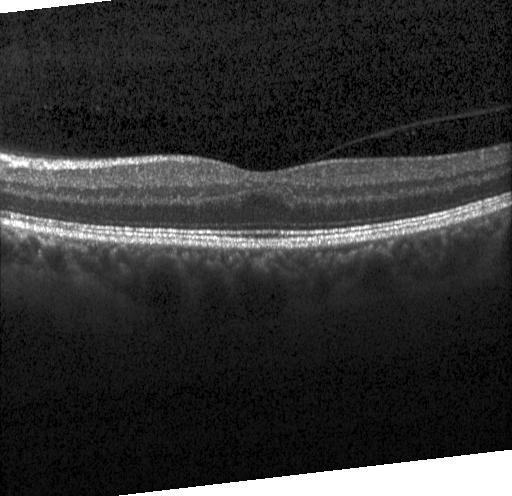 OCT line scan — Dx: no choroidal neovascularization, no diabetic macular edema, and no drusen.